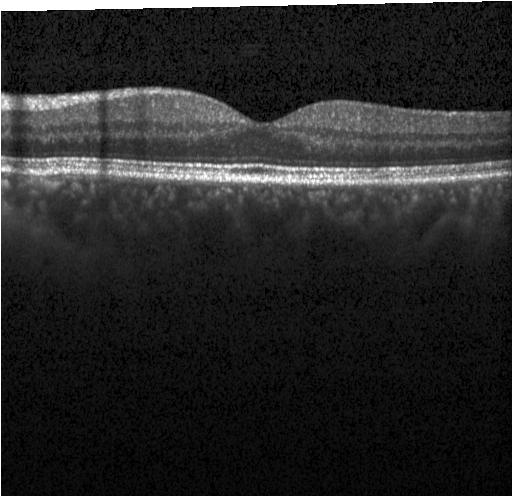

Retinal OCT B-scan. Fovea-centered. Heidelberg Spectralis OCT system. SD-OCT.
The scan shows no evidence of CNV, DME, or drusen.